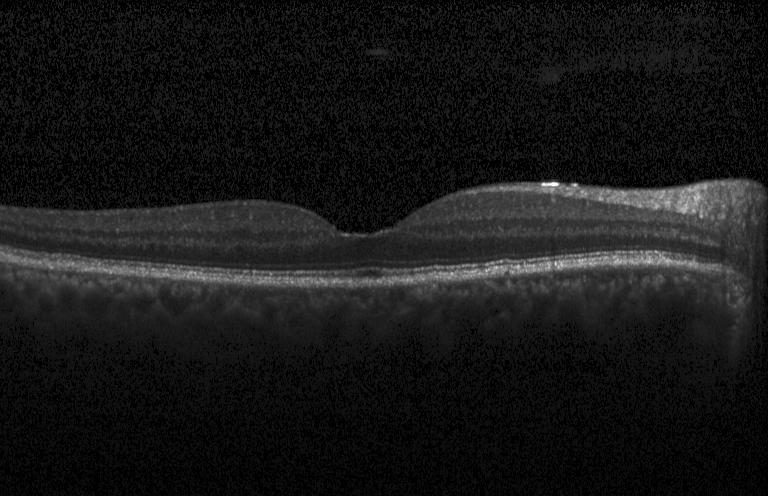

Diagnosis: no CNV, no DME, and no drusen.